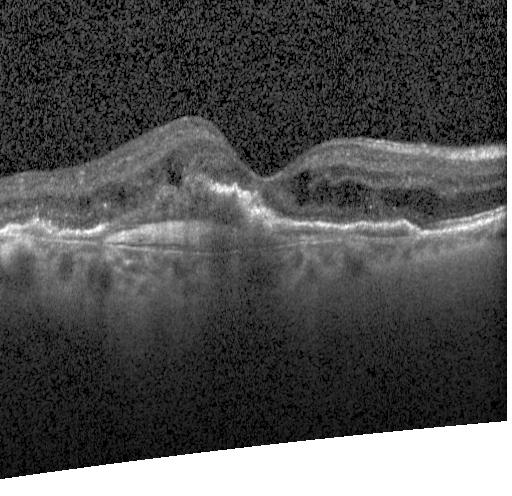

Retinal OCT B-scan — Diagnosis: choroidal neovascularization.